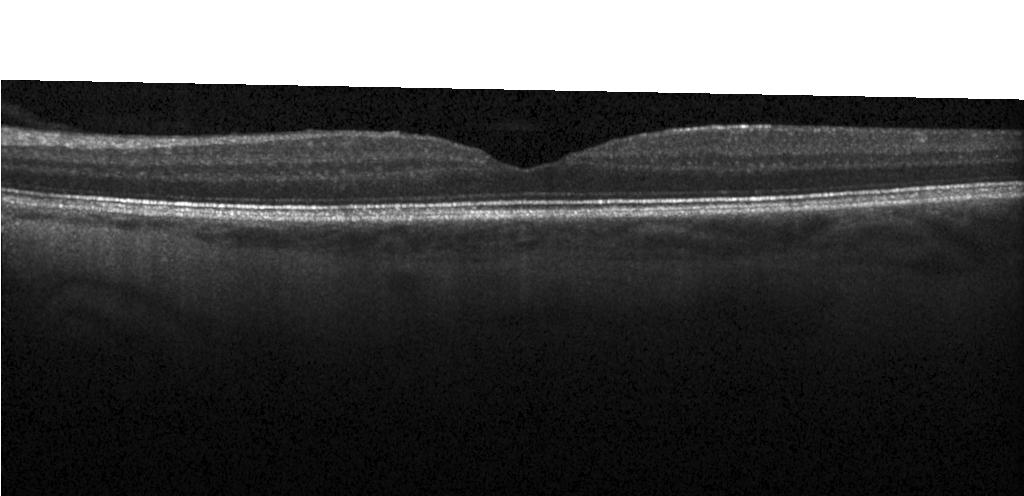 Retinal OCT cross-section — The scan shows no choroidal neovascularization, no diabetic macular edema, and no drusen.